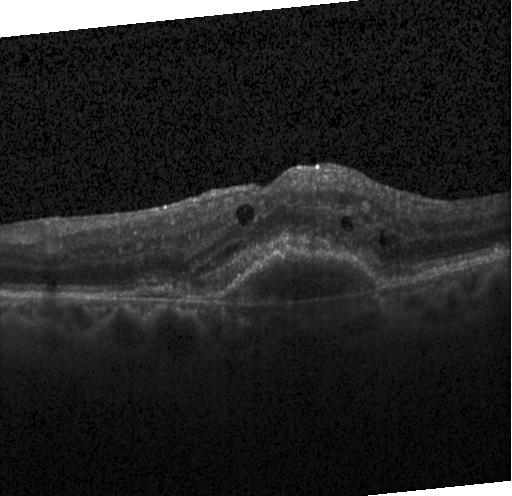 Finding: a choroidal neovascular membrane.